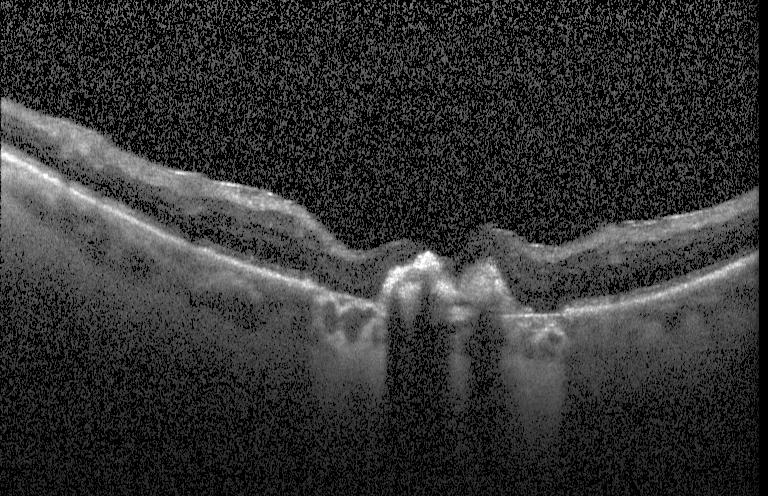 OCT line scan; centered on the fovea; spectral-domain OCT. OCT finding: CNV.